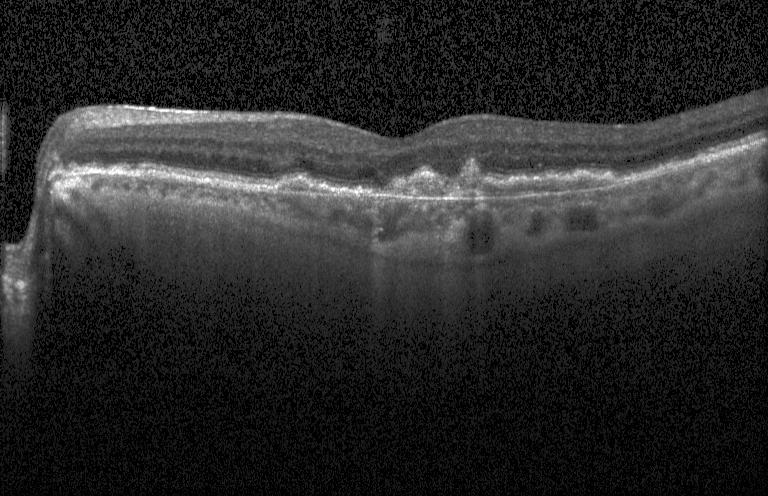 Optical coherence tomography B-scan. OCT finding: a choroidal neovascular membrane.